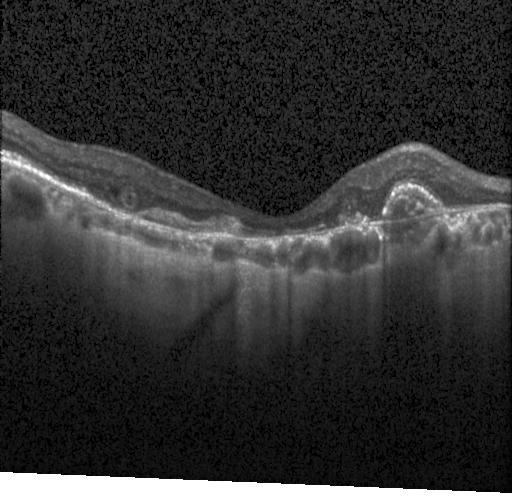
OCT line scan. Fovea-centered. SD-OCT. Instrument: Heidelberg Spectralis.
A choroidal neovascular membrane.